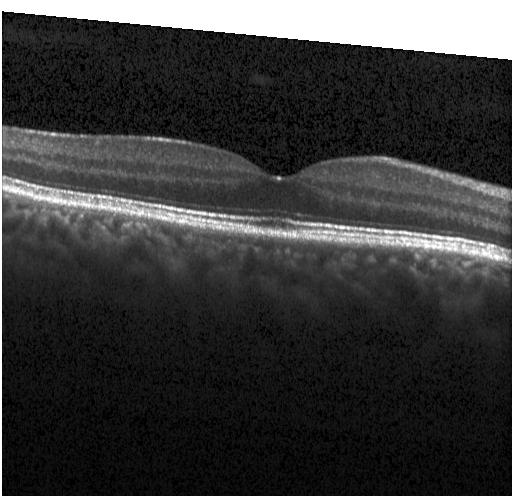

OCT line scan; SD-OCT. Impression: no choroidal neovascularization, diabetic macular edema, or drusen.